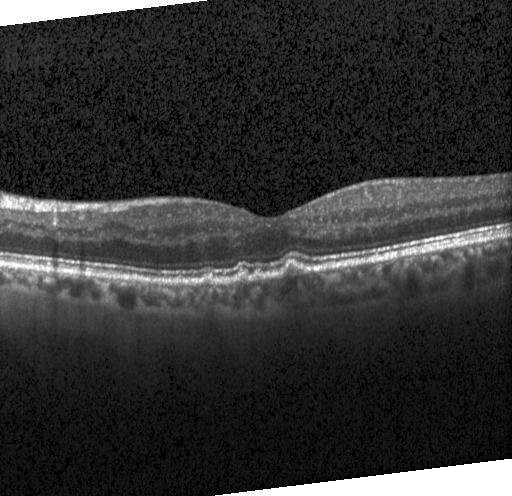
Optical coherence tomography scan. Diagnosis: drusen.